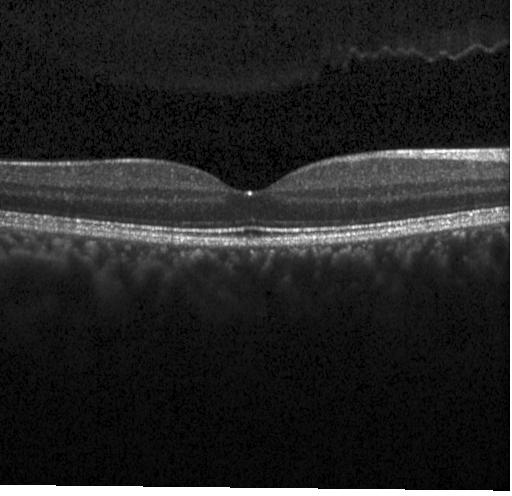
Impression: neither choroidal neovascularization, diabetic macular edema, nor drusen.